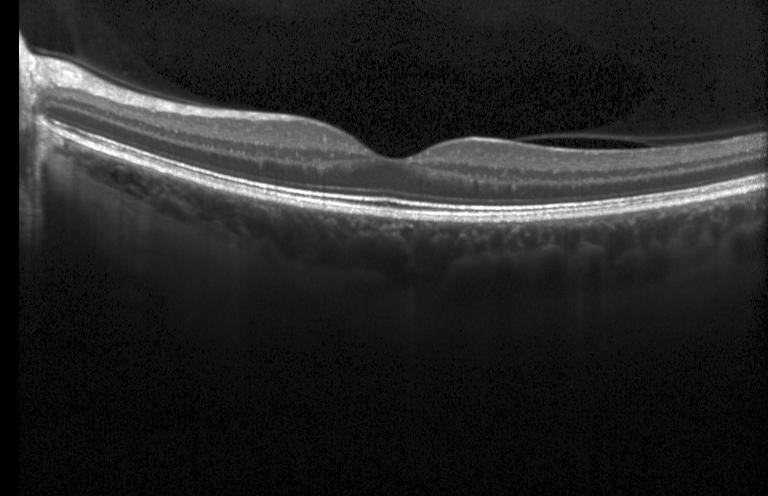 Optical coherence tomography scan.
Finding: neither choroidal neovascularization, diabetic macular edema, nor drusen.